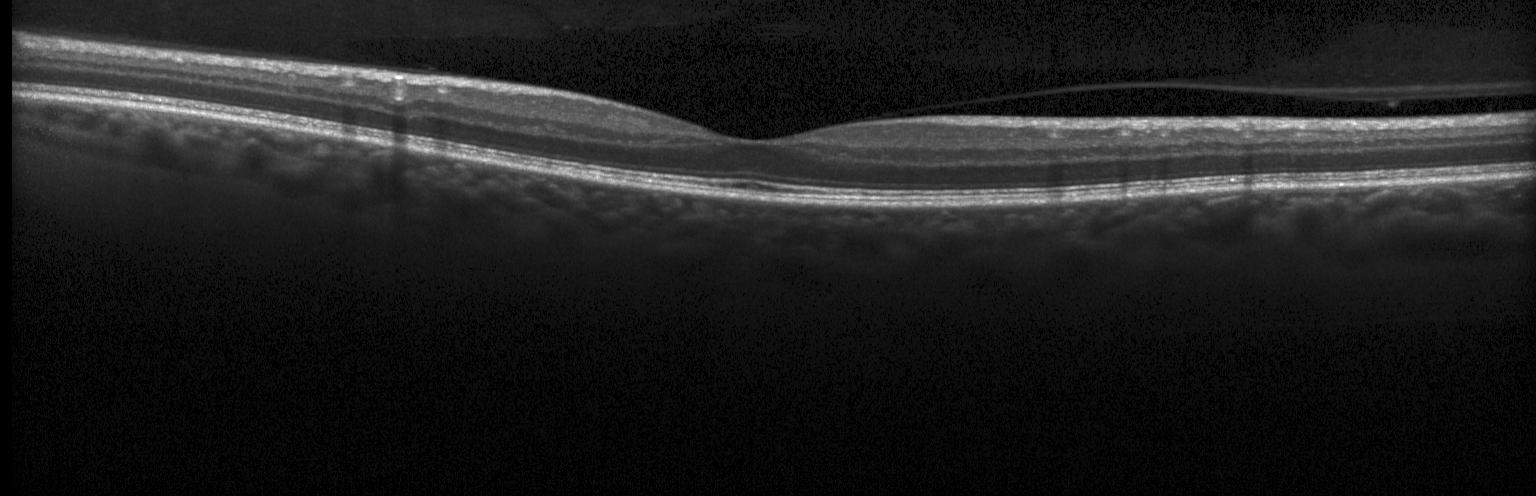

Optical coherence tomography scan.
Macular OCT: no choroidal neovascularization, no diabetic macular edema, and no drusen.